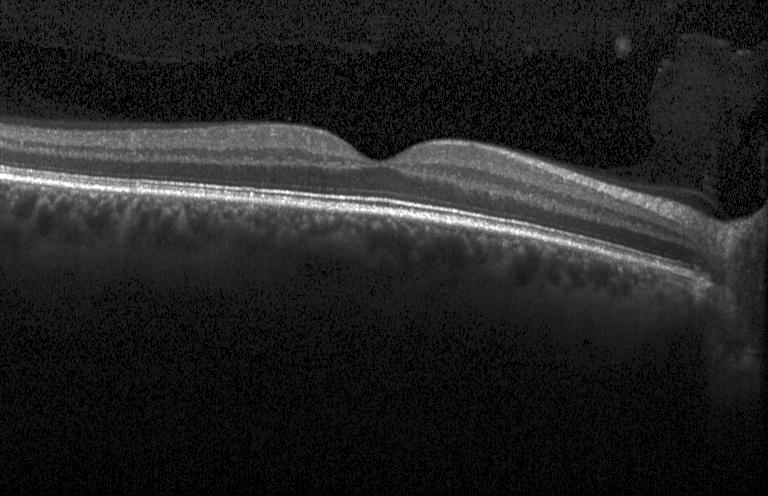
Retinal OCT B-scan
Finding: neither CNV, DME, nor drusen.